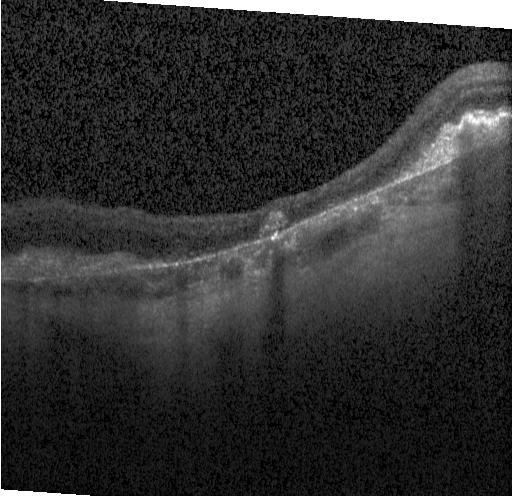 Macular scan. Optical coherence tomography scan.
This B-scan demonstrates a choroidal neovascular membrane.